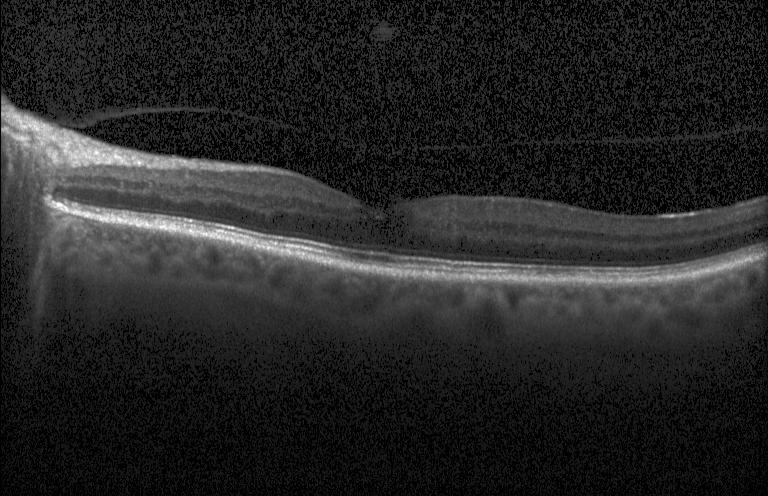

Instrument: Heidelberg Spectralis, spectral-domain OCT, retinal OCT cross-section. Finding: no choroidal neovascularization, no diabetic macular edema, and no drusen.